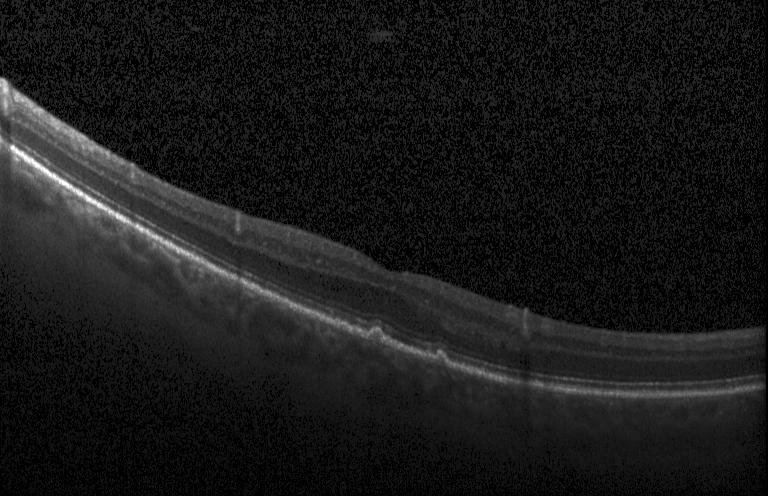
Macular OCT: multiple drusen.